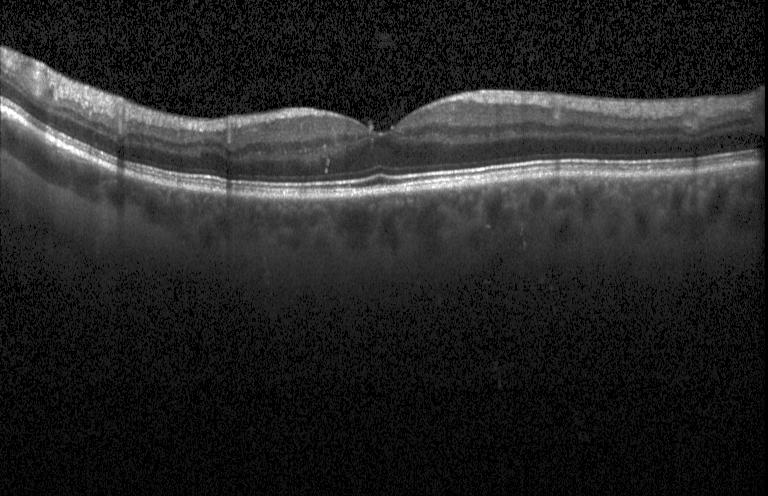 Instrument: Heidelberg Spectralis. OCT line scan
The scan shows neither CNV, DME, nor drusen.